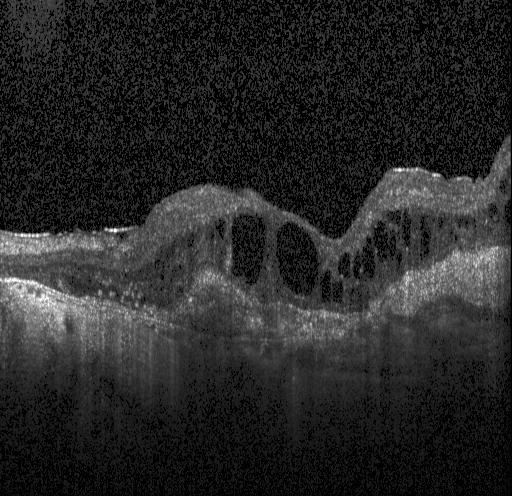

Retinal OCT B-scan. Heidelberg Spectralis OCT system. SD-OCT
Finding: a choroidal neovascular membrane.